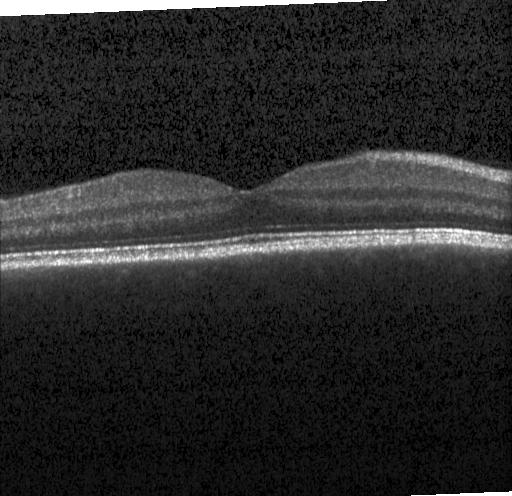

OCT line scan, SD-OCT, Heidelberg Spectralis, through the macula
Finding: no evidence of CNV, DME, or drusen.